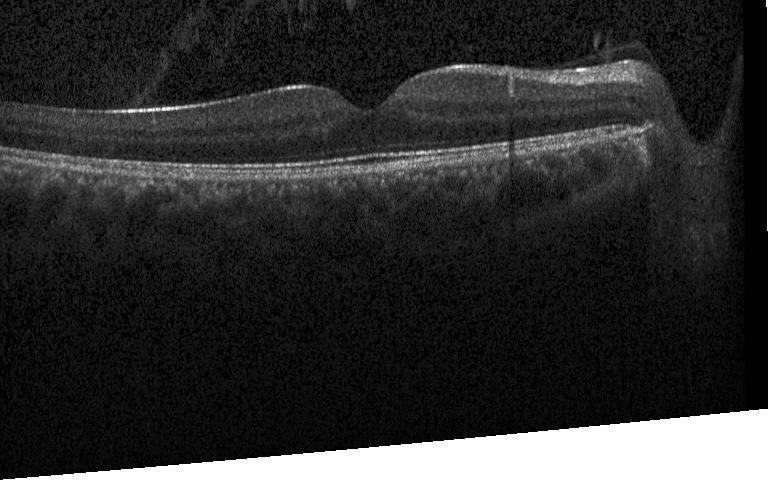
Impression: no choroidal neovascularization, diabetic macular edema, or drusen.